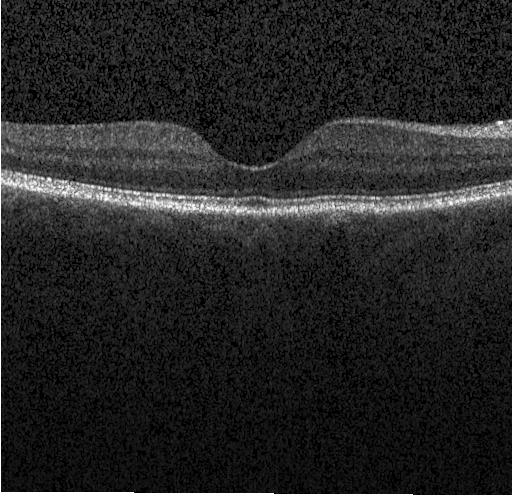

Spectral-domain OCT B-scan: no CNV, DME, or drusen.